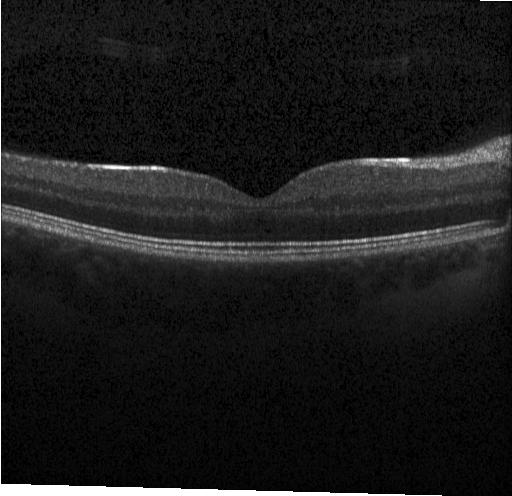
Optical coherence tomography scan, spectral-domain optical coherence tomography — The scan shows no choroidal neovascularization, no diabetic macular edema, and no drusen.